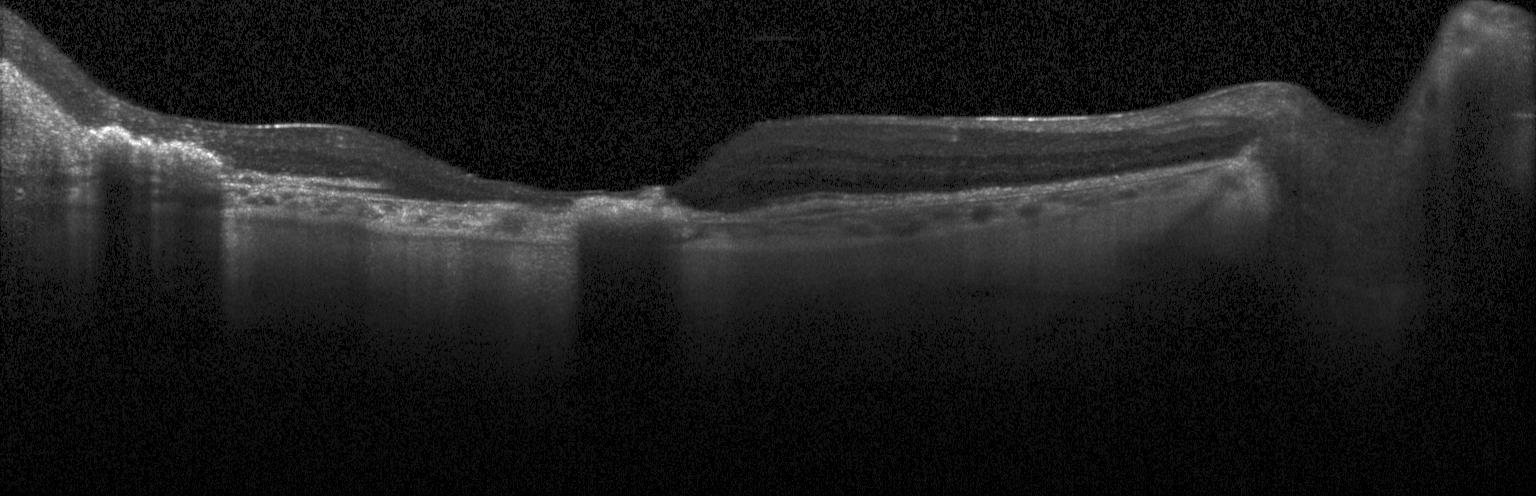

Macular OCT: CNV.